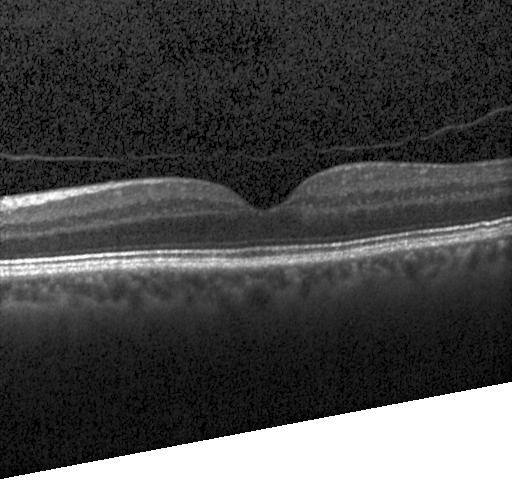

Through the macula. Optical coherence tomography scan
Assessment: no choroidal neovascularization, diabetic macular edema, or drusen.